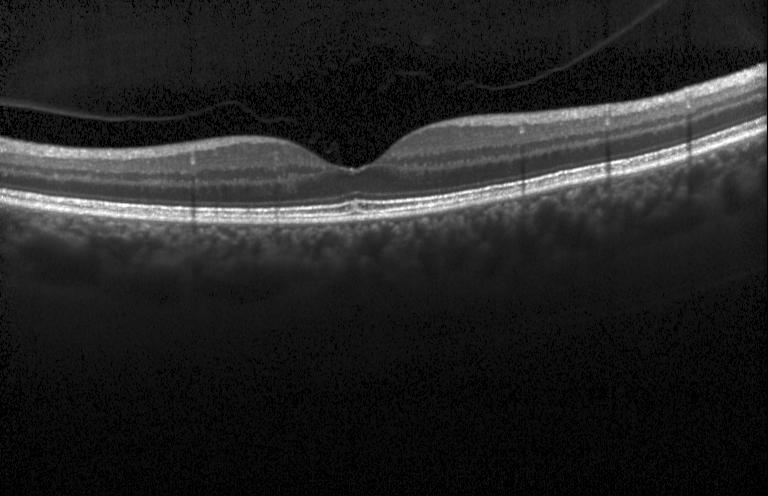
Acquired on a Heidelberg Spectralis. SD-OCT. Optical coherence tomography B-scan — Assessment: no evidence of choroidal neovascularization, diabetic macular edema, or drusen.